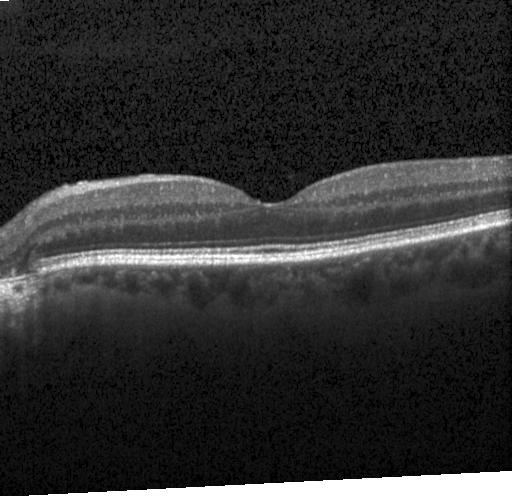
Optical coherence tomography scan
No choroidal neovascularization, no diabetic macular edema, and no drusen.